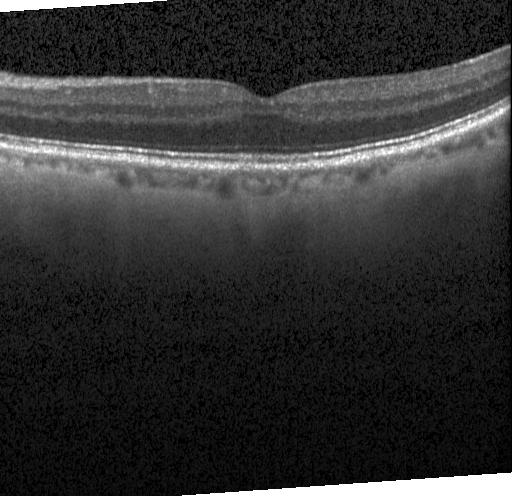 Retinal OCT B-scan, SD-OCT
This B-scan demonstrates no choroidal neovascularization, diabetic macular edema, or drusen.